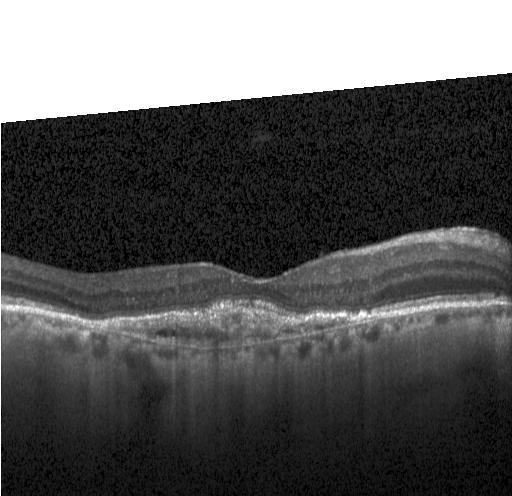

OCT scan showing a choroidal neovascular membrane.